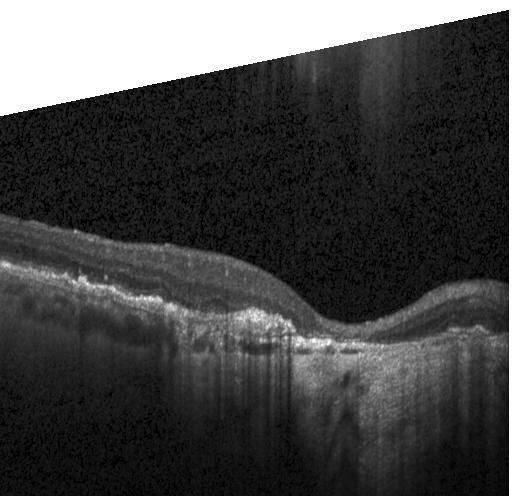
Optical coherence tomography B-scan — Dx: a choroidal neovascular membrane.